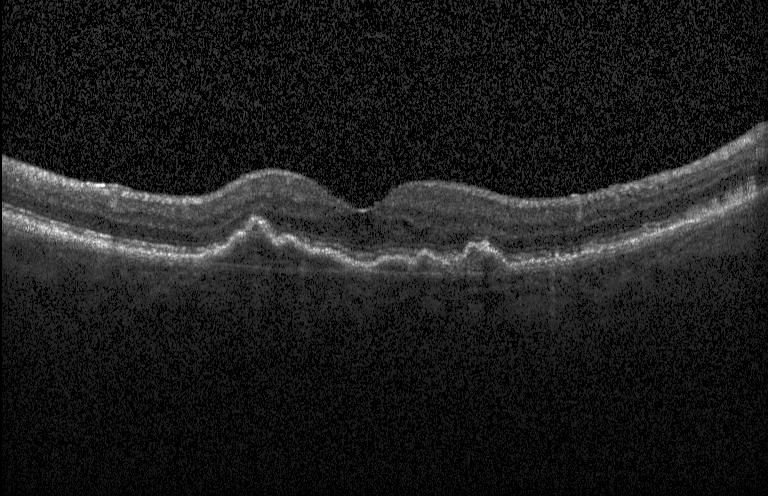

OCT scan showing a choroidal neovascular membrane.